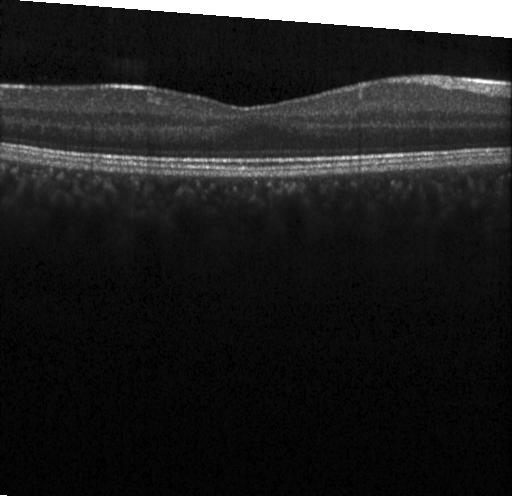

Retinal OCT cross-section showing no choroidal neovascularization, no diabetic macular edema, and no drusen.